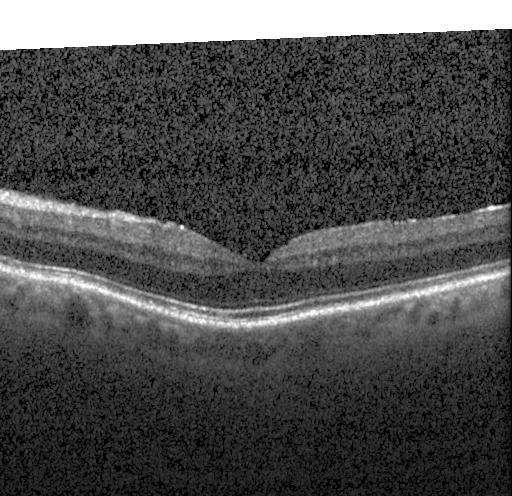

Heidelberg Spectralis OCT system, optical coherence tomography scan, macular scan — The scan shows no evidence of choroidal neovascularization, diabetic macular edema, or drusen.